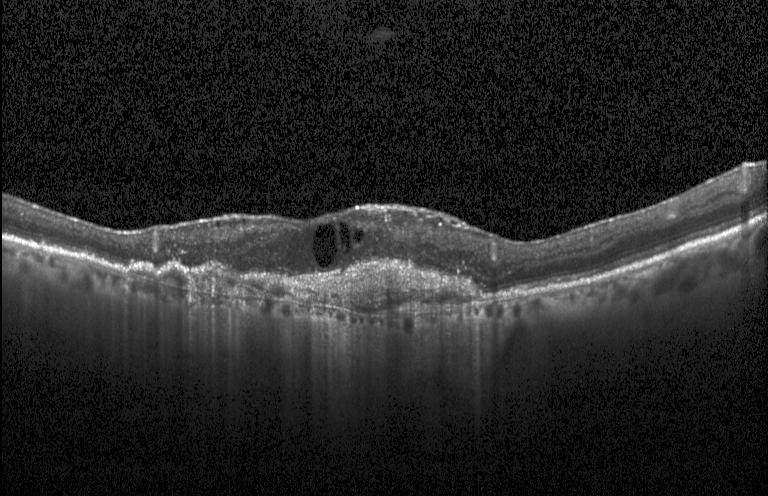

This B-scan demonstrates choroidal neovascularization (CNV).